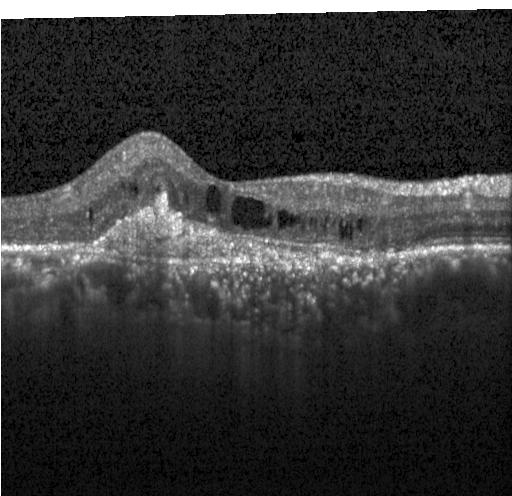
Fovea-centered · spectral-domain optical coherence tomography · instrument: Heidelberg Spectralis · OCT line scan.
The scan shows a choroidal neovascular membrane.